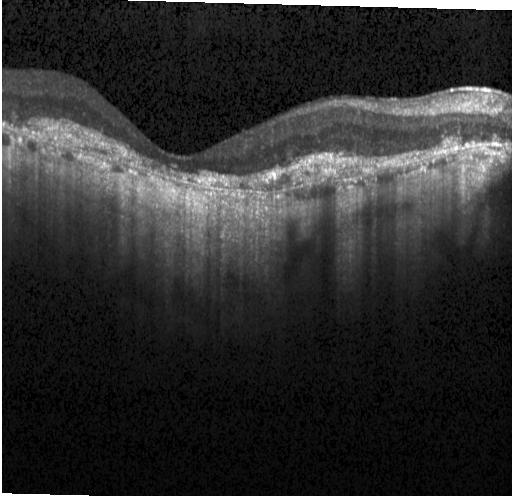
Optical coherence tomography B-scan; spectral-domain optical coherence tomography — Impression: a choroidal neovascular membrane.